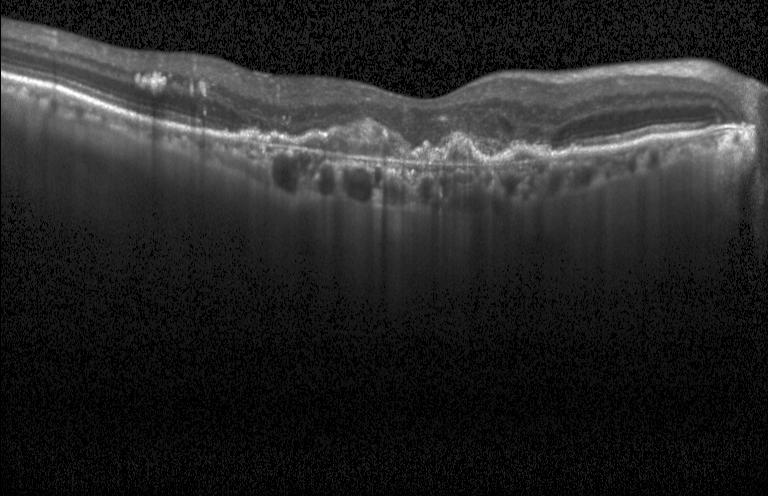 OCT B-scan showing choroidal neovascularization (CNV).